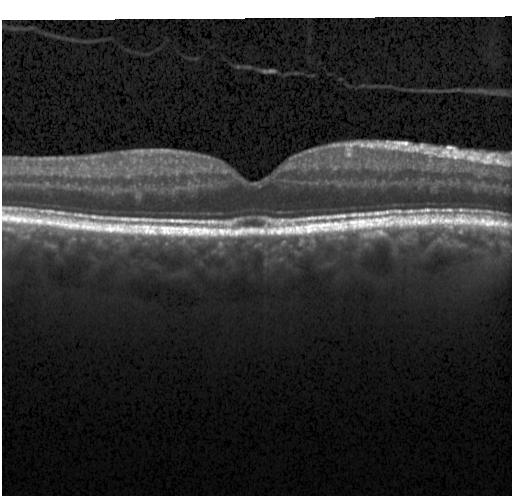 Spectral-domain OCT B-scan: neither choroidal neovascularization, diabetic macular edema, nor drusen.